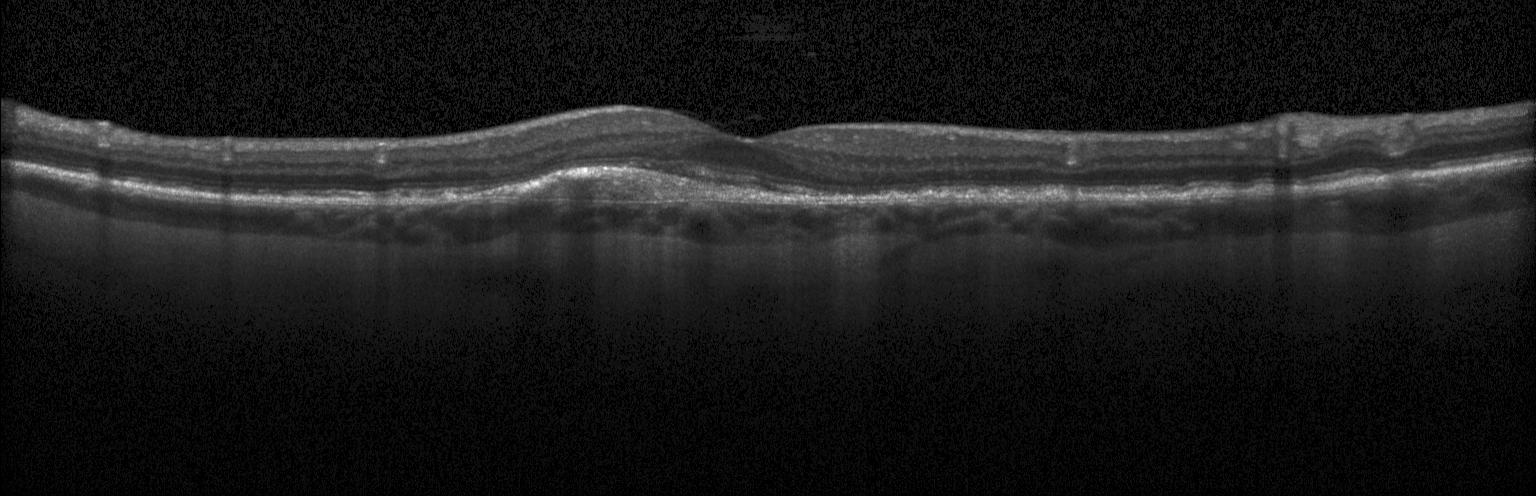

Impression: a choroidal neovascular membrane.